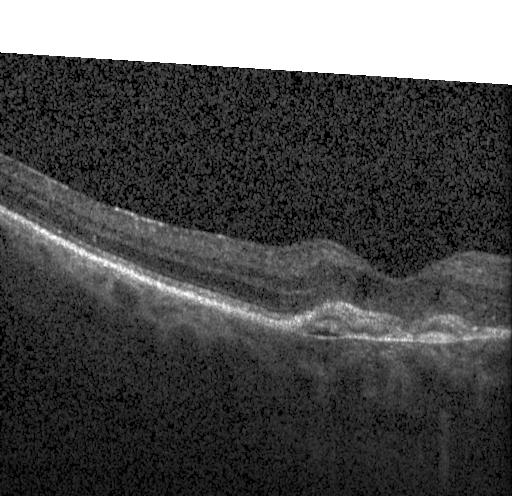
Impression: choroidal neovascularization (CNV).